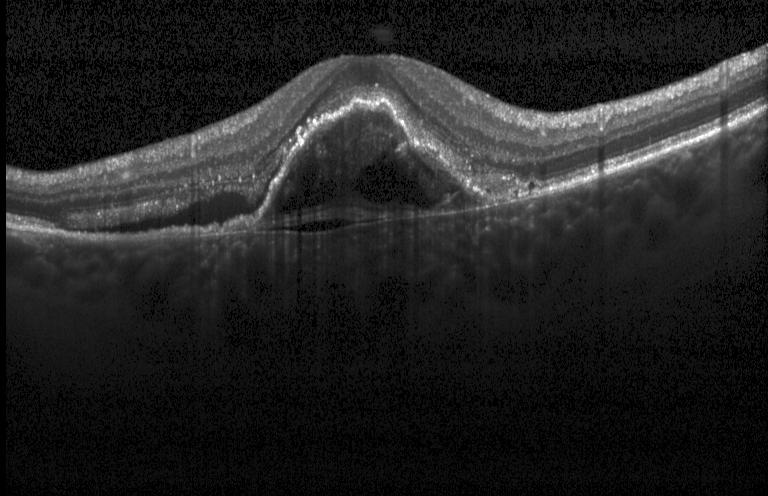 Impression: a choroidal neovascular membrane.